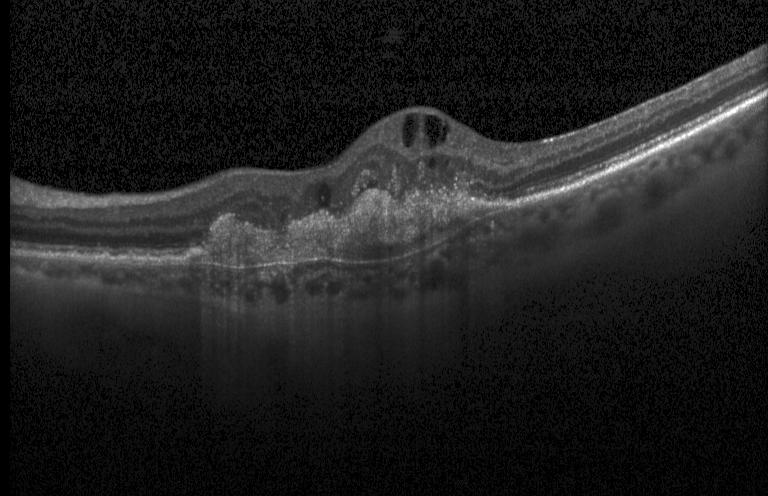

Optical coherence tomography B-scan — Assessment: a choroidal neovascular membrane.